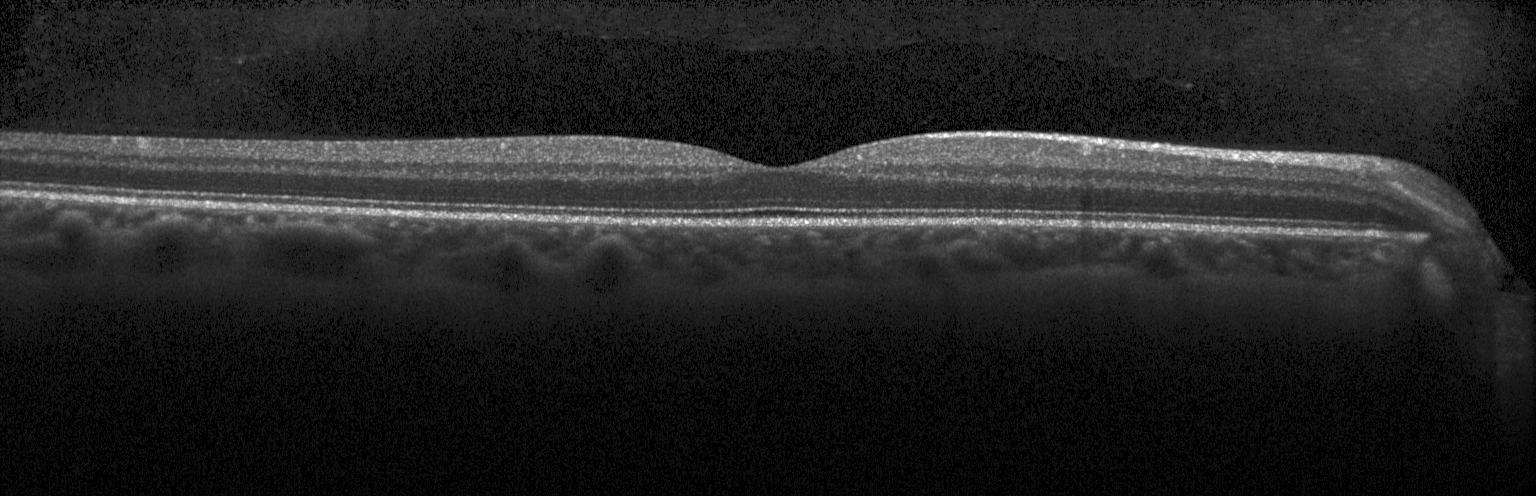

Fovea-centered, OCT B-scan, instrument: Heidelberg Spectralis. No evidence of CNV, DME, or drusen.